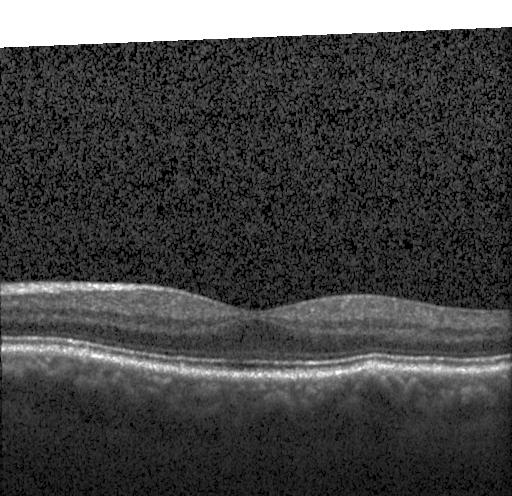

Instrument: Heidelberg Spectralis. Optical coherence tomography B-scan. This B-scan demonstrates no evidence of choroidal neovascularization, diabetic macular edema, or drusen.